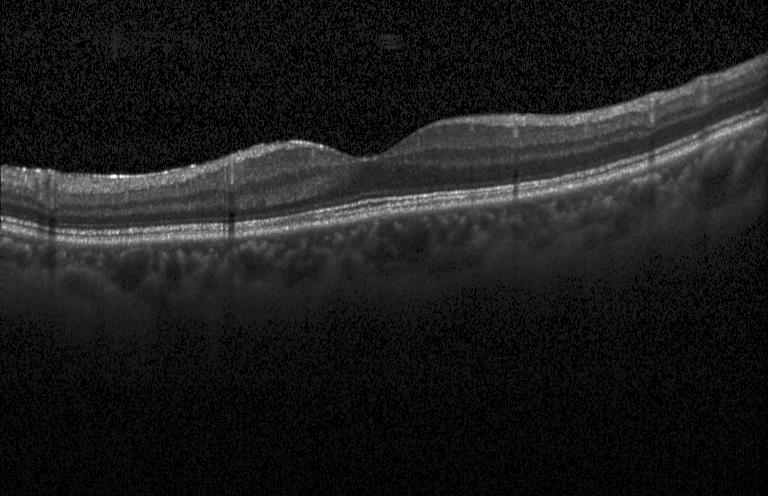
Through the macula · optical coherence tomography B-scan · spectral-domain optical coherence tomography — Impression: neither CNV, DME, nor drusen.